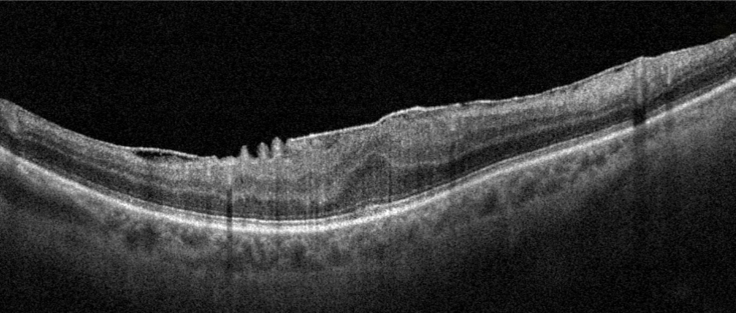 Retinal OCT cross-section. Macular OCT: epiretinal membrane.